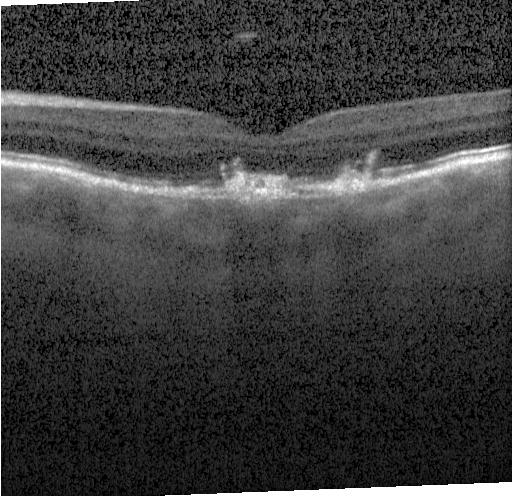 Retinal OCT cross-section showing a choroidal neovascular membrane.